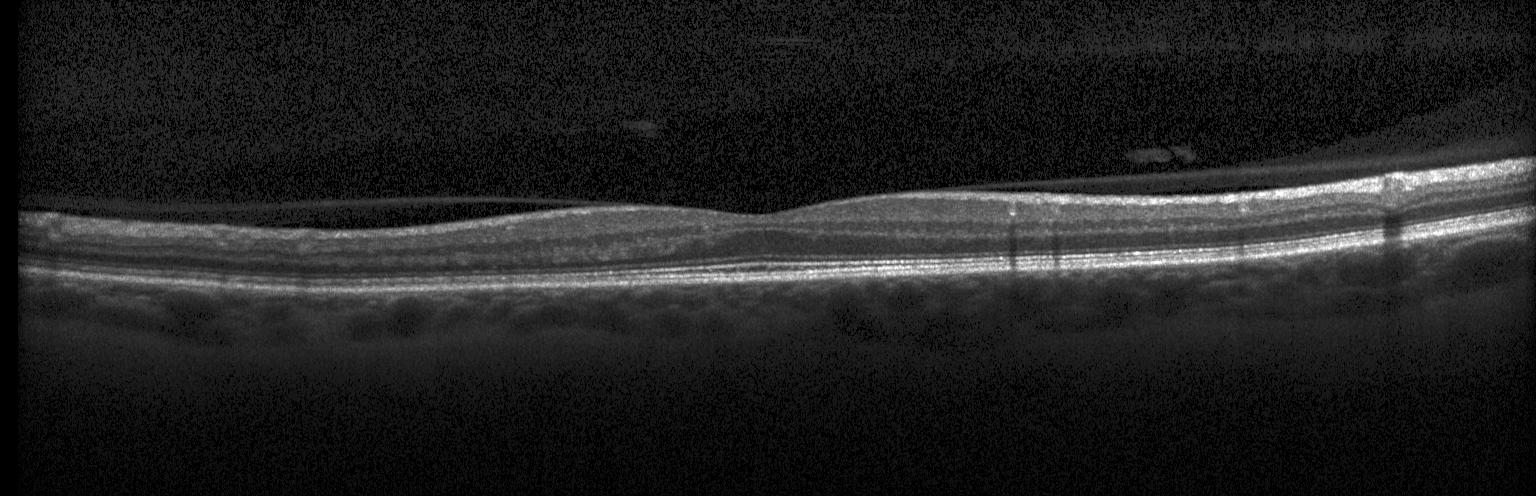 Macular OCT: neither choroidal neovascularization, diabetic macular edema, nor drusen.